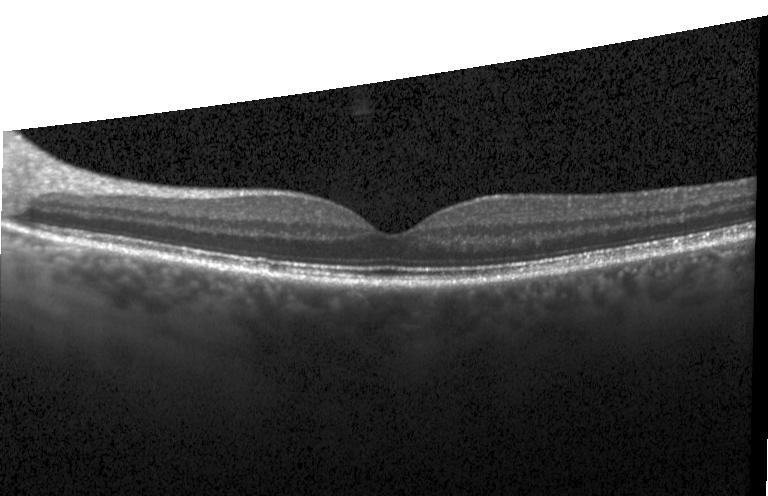 Finding: no evidence of CNV, DME, or drusen.